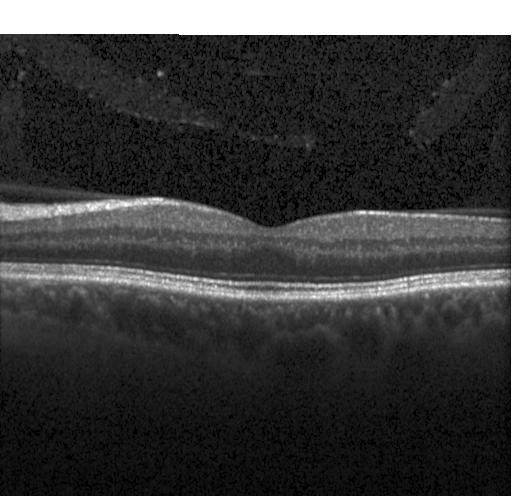 Retinal OCT cross-section showing neither choroidal neovascularization, diabetic macular edema, nor drusen.